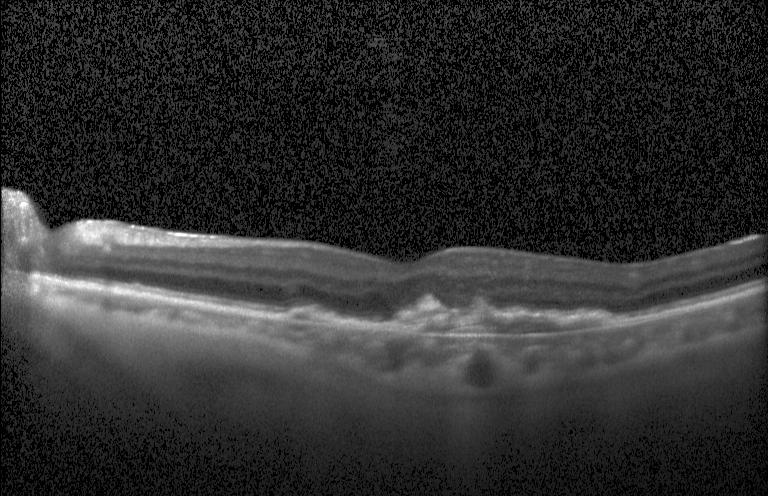 OCT B-scan — Diagnosis: CNV.